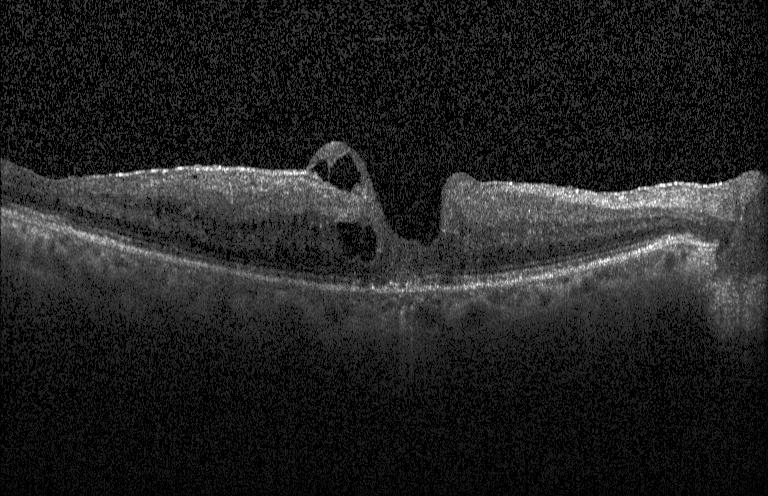
This B-scan demonstrates diabetic macular edema (DME).